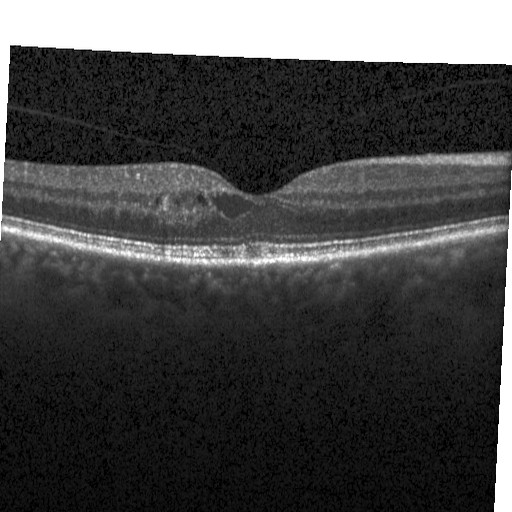
Centered on the fovea, spectral-domain OCT, acquired on a Heidelberg Spectralis, optical coherence tomography scan
Finding: DME.